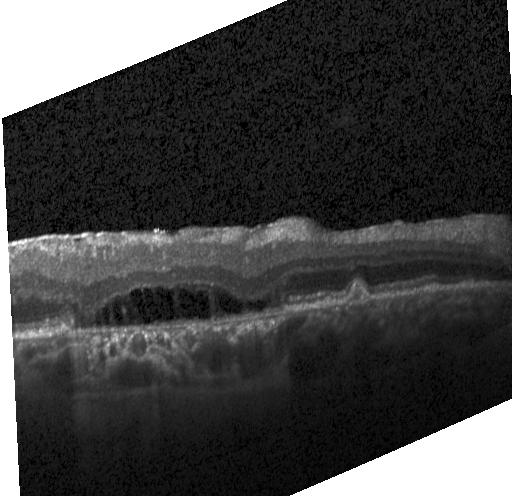
The scan shows a choroidal neovascular membrane.